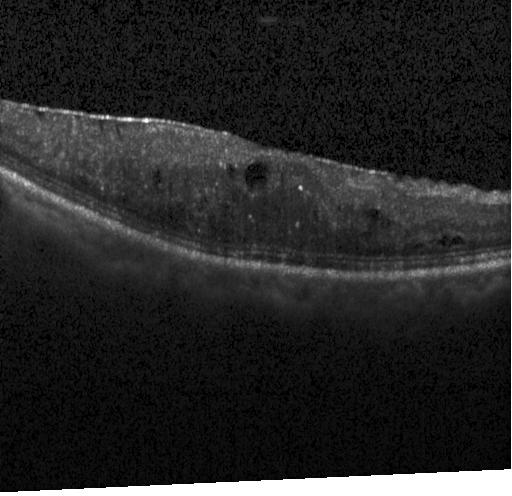 Spectral-domain OCT. OCT line scan. Heidelberg Spectralis.
Finding: diabetic macular edema.